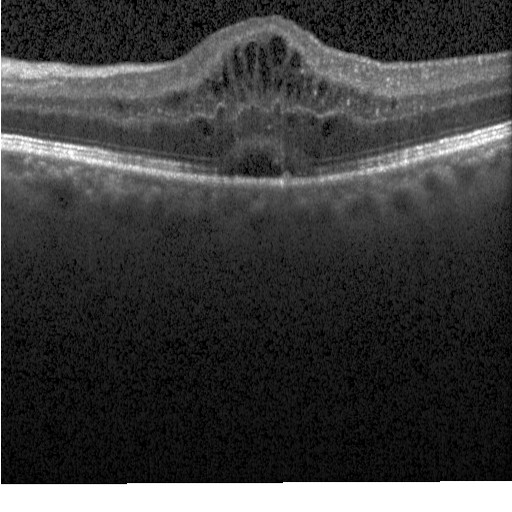 Diagnosis: diabetic macular edema (DME).